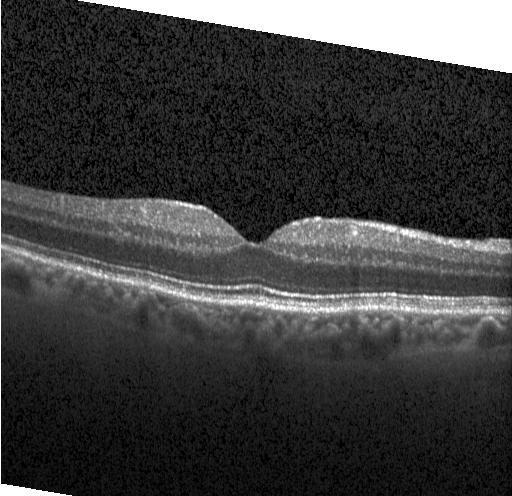 This B-scan demonstrates no evidence of choroidal neovascularization, diabetic macular edema, or drusen.